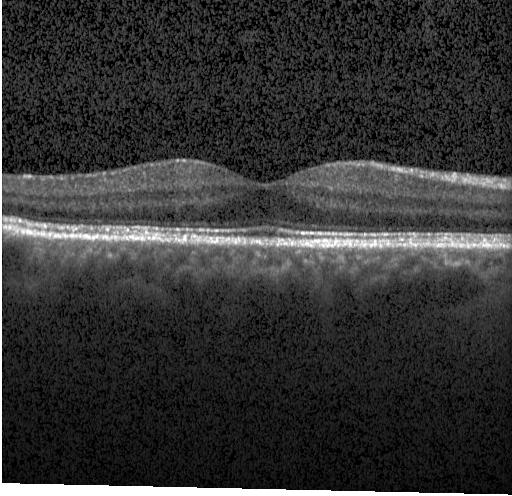

Retinal OCT cross-section showing no choroidal neovascularization, diabetic macular edema, or drusen.